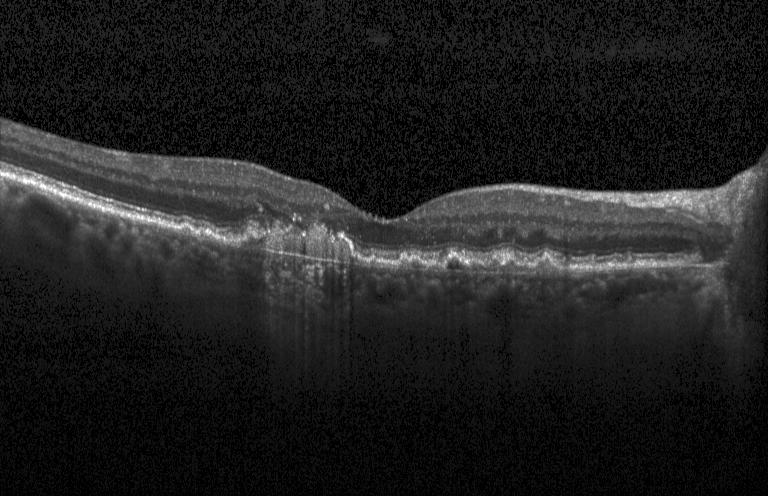 A choroidal neovascular membrane.